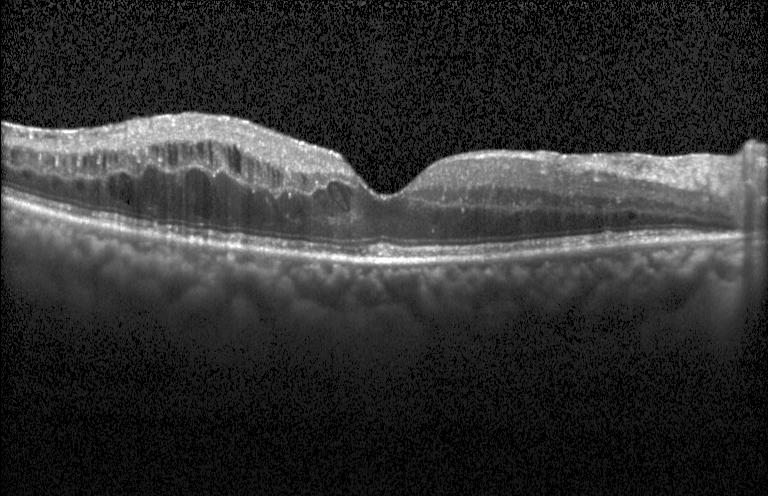

Macular OCT demonstrating diabetic macular edema (DME).